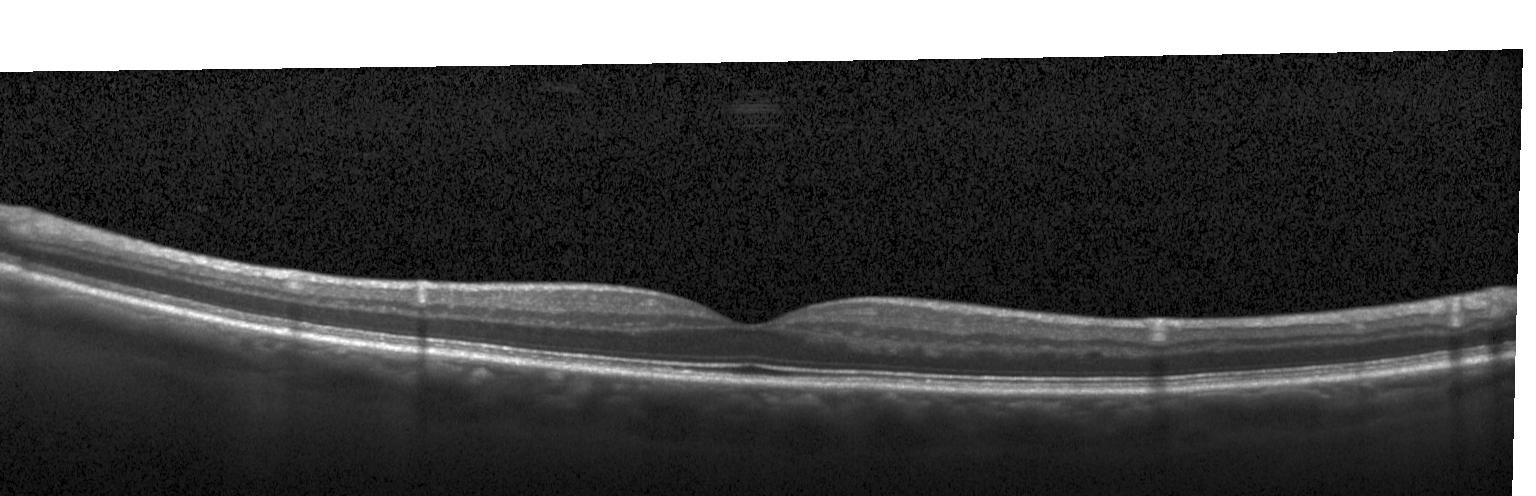

OCT B-scan. Horizontal scan through the fovea. Heidelberg Spectralis OCT system.
Dx: no CNV, DME, or drusen.